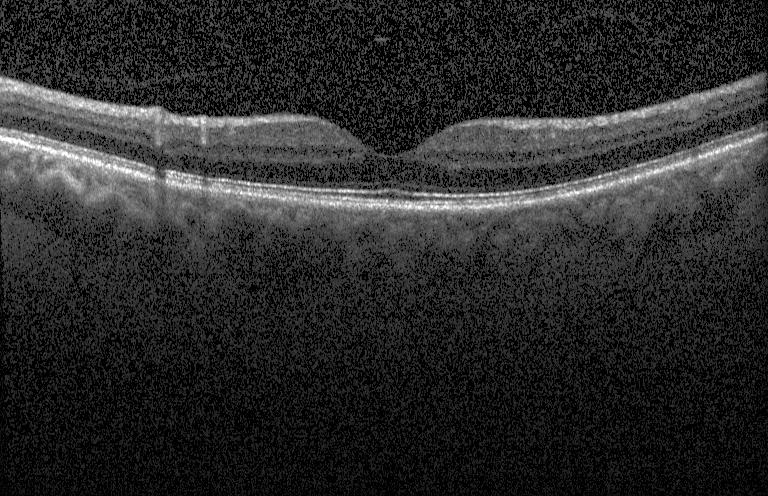
Optical coherence tomography B-scan.
Macular OCT: no evidence of choroidal neovascularization, diabetic macular edema, or drusen.